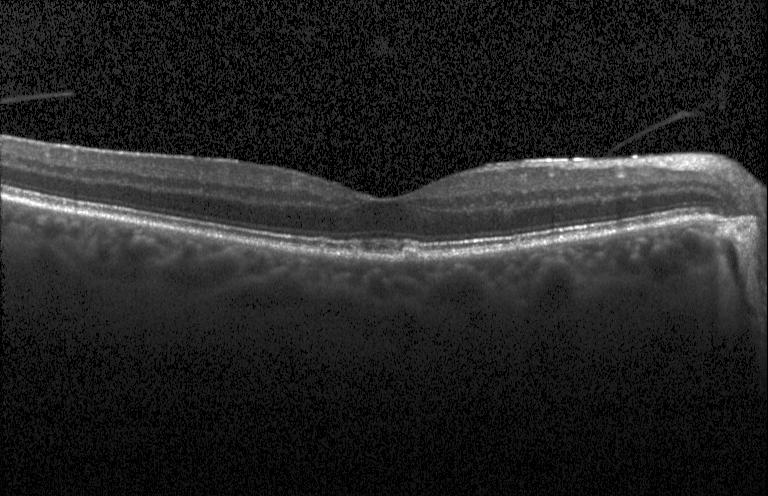

OCT scan showing sub-RPE drusenoid deposits.